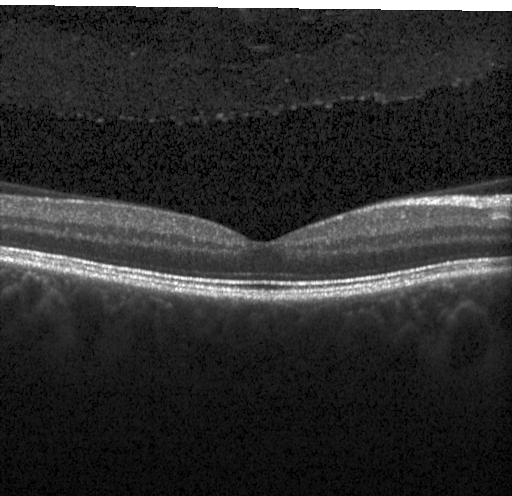
OCT finding: neither CNV, DME, nor drusen.